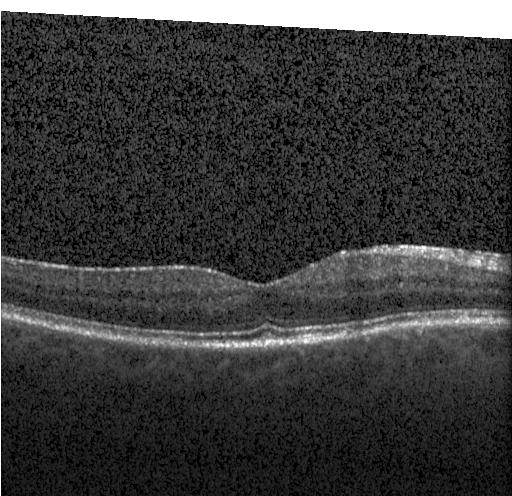
Diagnosis: no CNV, DME, or drusen.